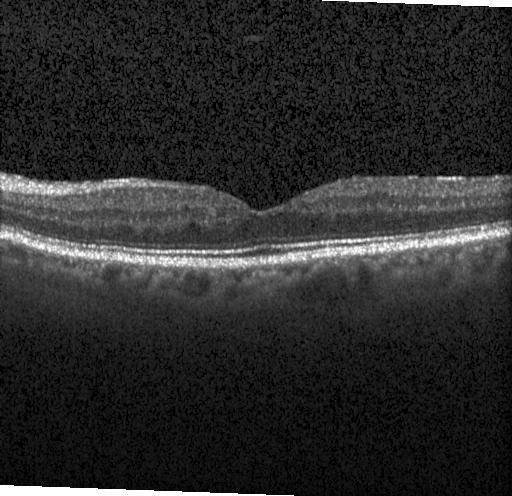 Spectral-domain OCT B-scan: no choroidal neovascularization, no diabetic macular edema, and no drusen.